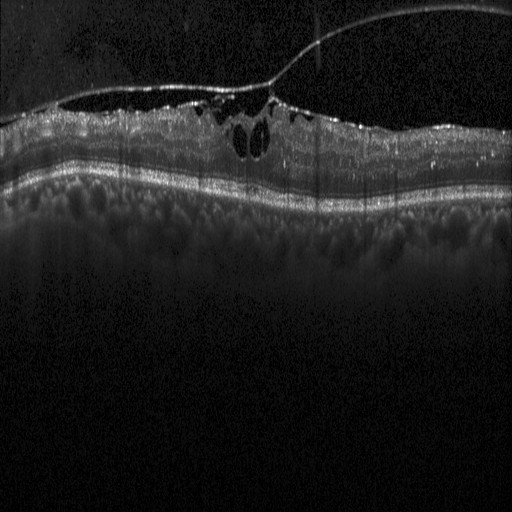
Heidelberg Spectralis OCT system · optical coherence tomography scan · spectral-domain optical coherence tomography
Dx: diabetic macular edema (DME).